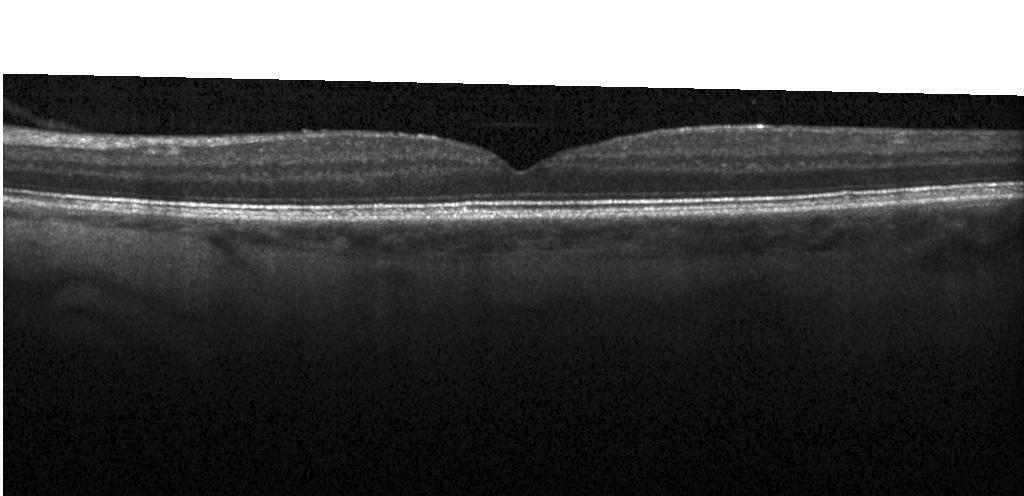
OCT line scan · fovea-centered · Heidelberg Spectralis · spectral-domain OCT.
Finding: no choroidal neovascularization, diabetic macular edema, or drusen.